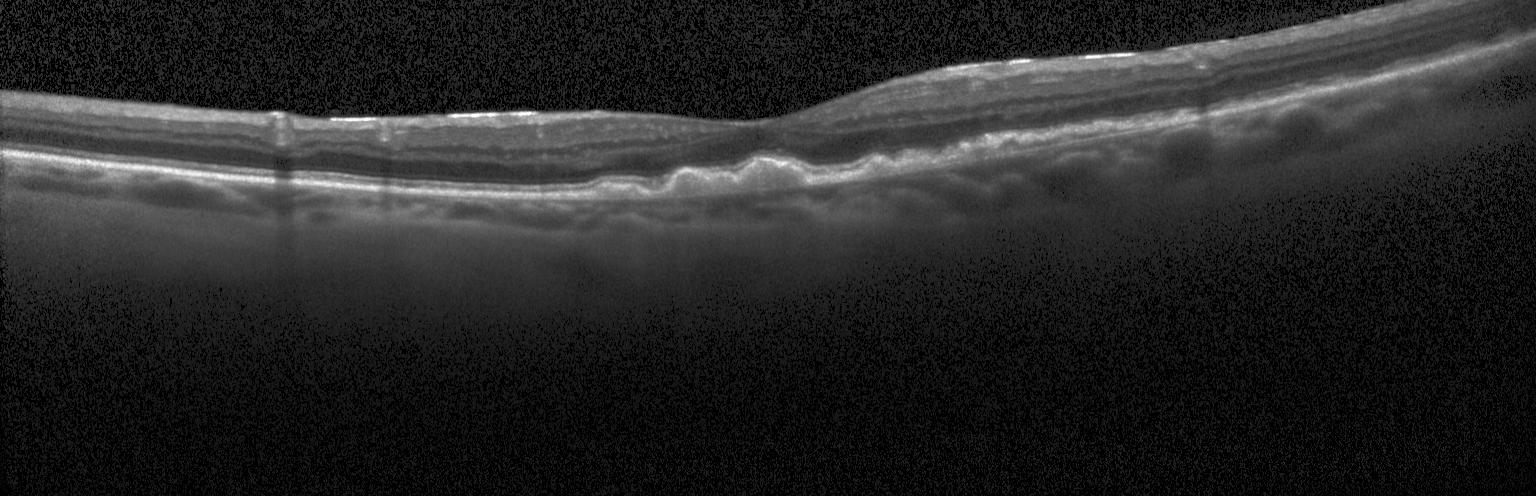 Optical coherence tomography scan. SD-OCT. Heidelberg Spectralis. The scan shows drusen.